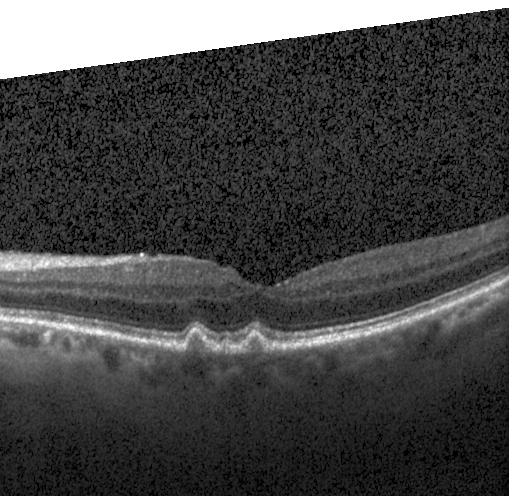

Finding: sub-RPE drusenoid deposits.